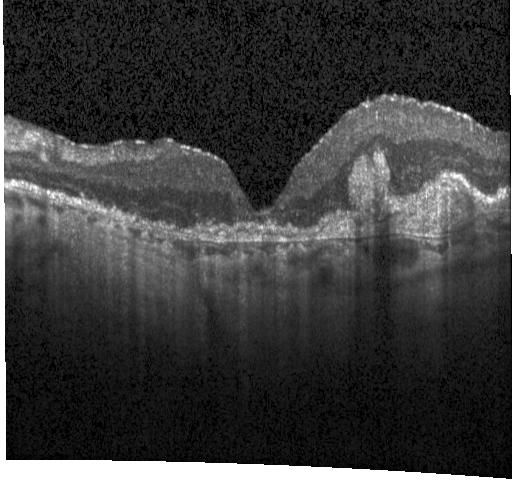
Macular scan. SD-OCT. Retinal OCT B-scan. Diagnosis: choroidal neovascularization (CNV).